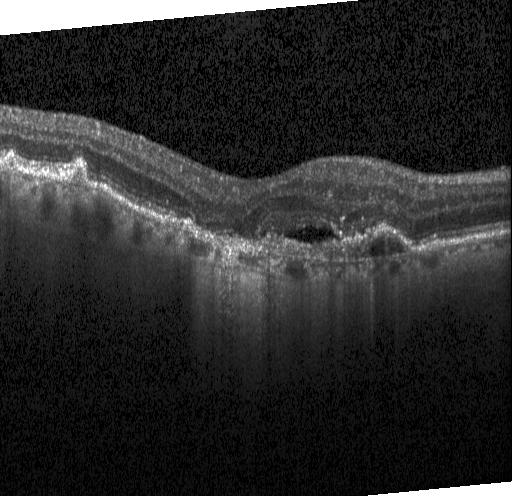
Finding: a choroidal neovascular membrane.